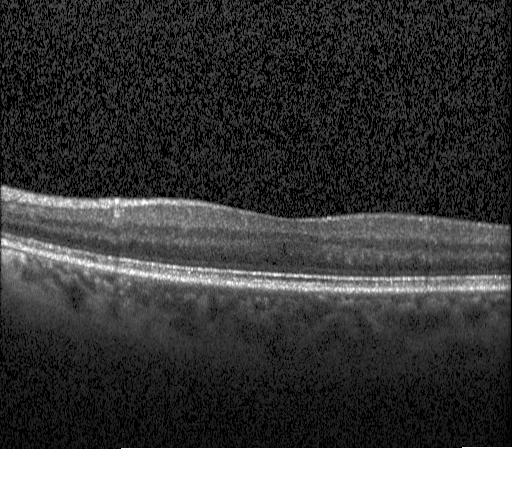 Instrument: Heidelberg Spectralis, OCT B-scan, spectral-domain OCT
Assessment: no CNV, DME, or drusen.